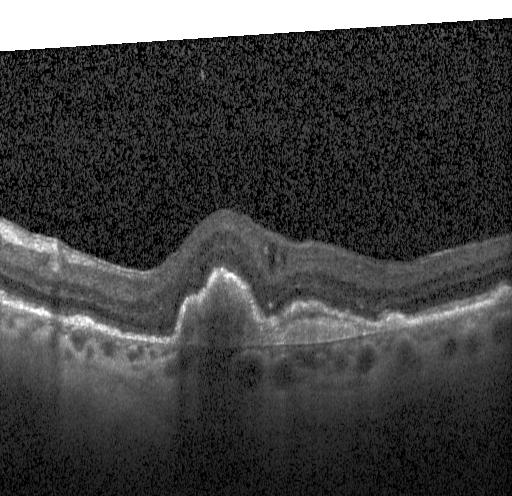 Optical coherence tomography scan
Choroidal neovascularization.